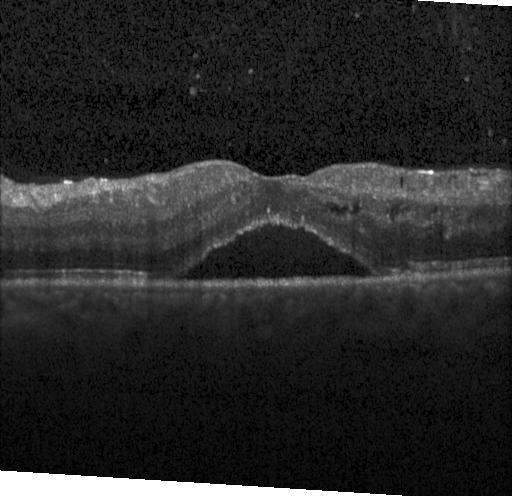

Finding: diabetic macular edema (DME).